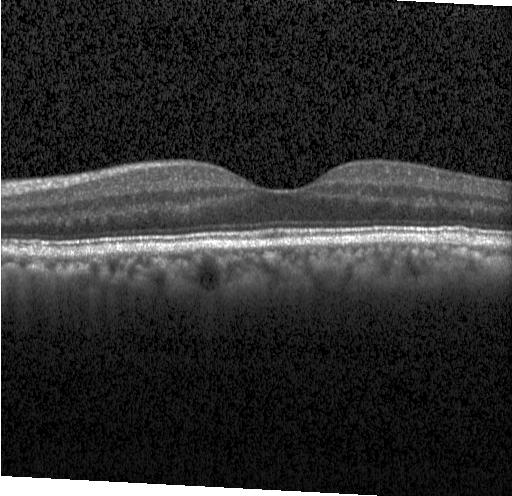
Finding: neither CNV, DME, nor drusen.